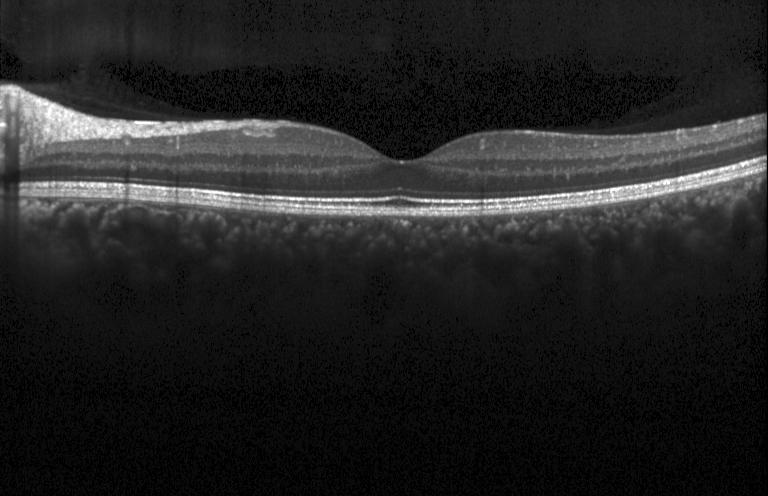

No CNV, no DME, and no drusen.